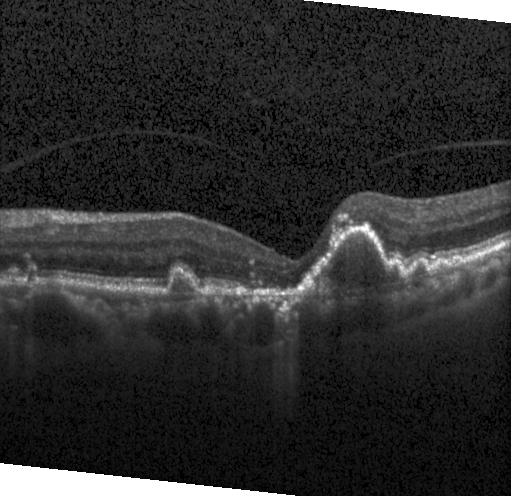

Optical coherence tomography scan; spectral-domain optical coherence tomography. This B-scan demonstrates a choroidal neovascular membrane.